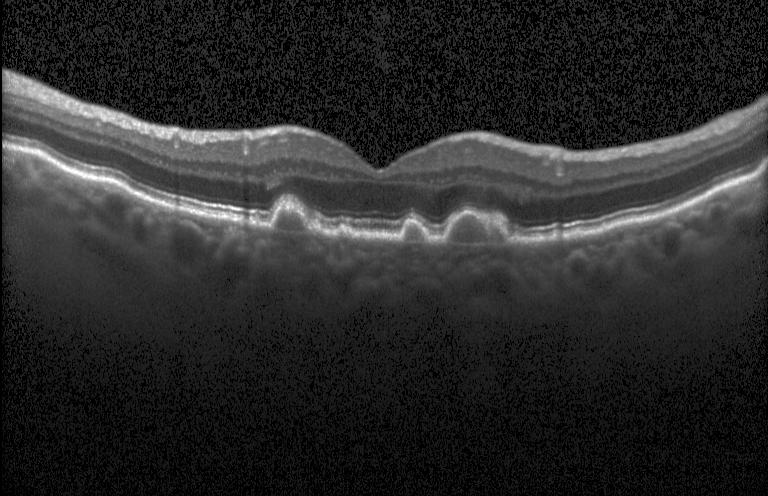
Retinal OCT B-scan; Heidelberg Spectralis OCT system; spectral-domain OCT
OCT finding: multiple drusen.